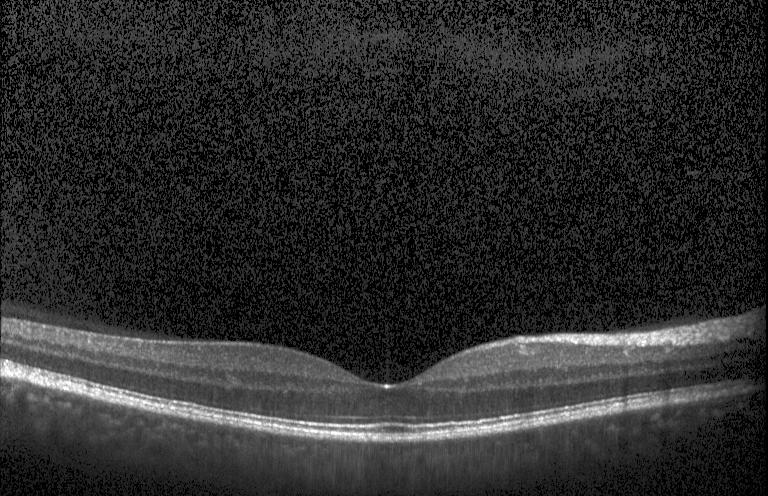 Macular scan, Heidelberg Spectralis OCT system, optical coherence tomography B-scan
This B-scan demonstrates no evidence of CNV, DME, or drusen.